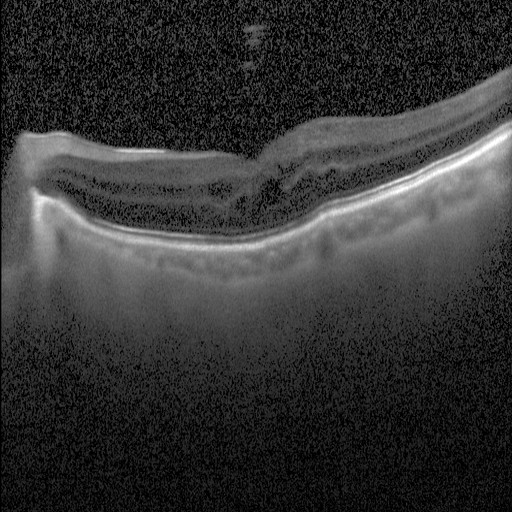

OCT B-scan showing diabetic macular edema.